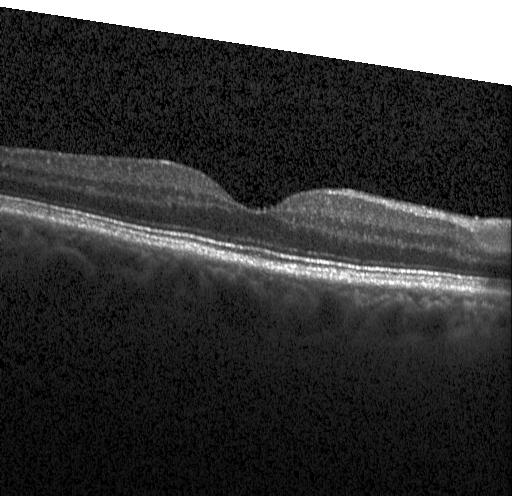
Spectral-domain OCT. Heidelberg Spectralis. OCT B-scan. Fovea-centered
Macular OCT: neither CNV, DME, nor drusen.